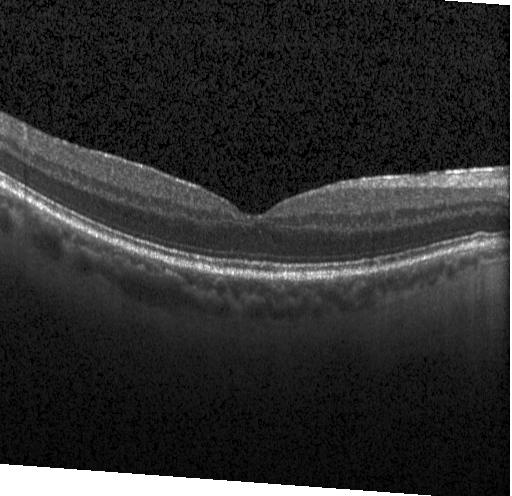

OCT line scan
Diagnosis: neither choroidal neovascularization, diabetic macular edema, nor drusen.